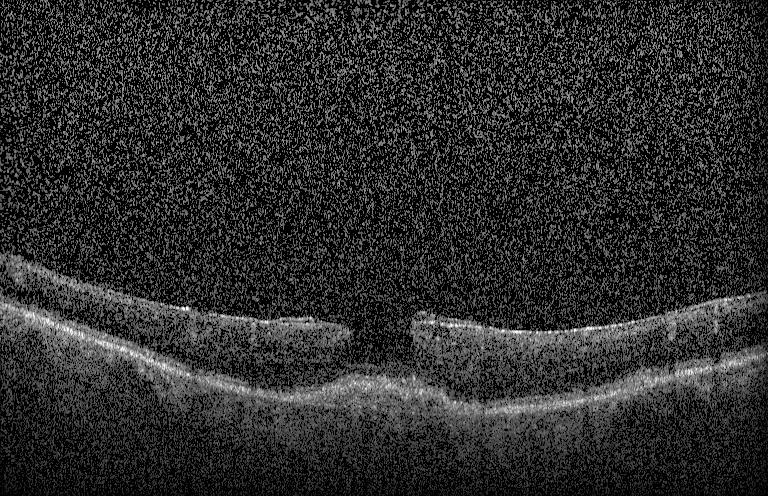 Macular OCT demonstrating CNV.